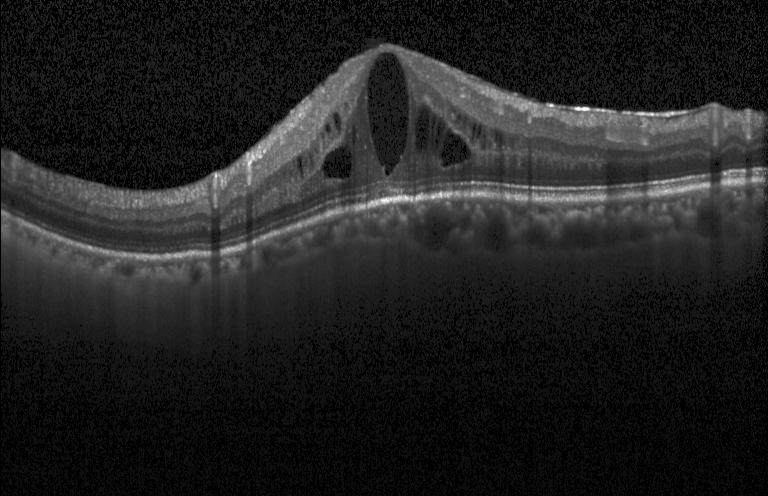 Spectral-domain optical coherence tomography, optical coherence tomography B-scan, acquired on a Heidelberg Spectralis, through the macula.
The scan shows diabetic macular edema.